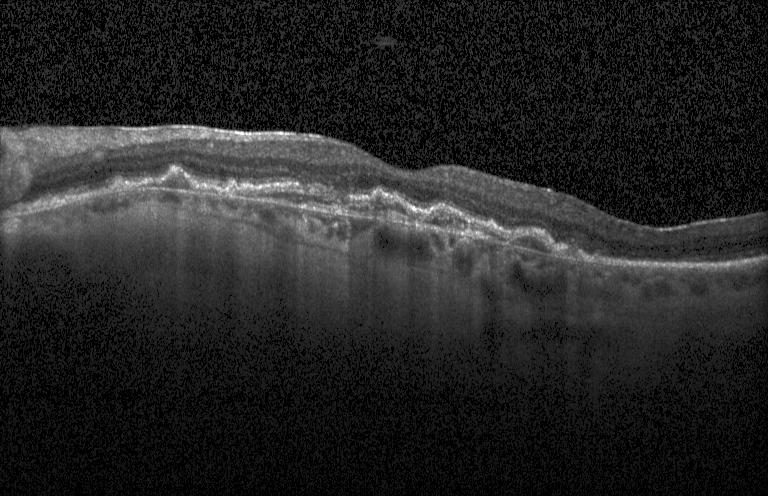 Impression: choroidal neovascularization.